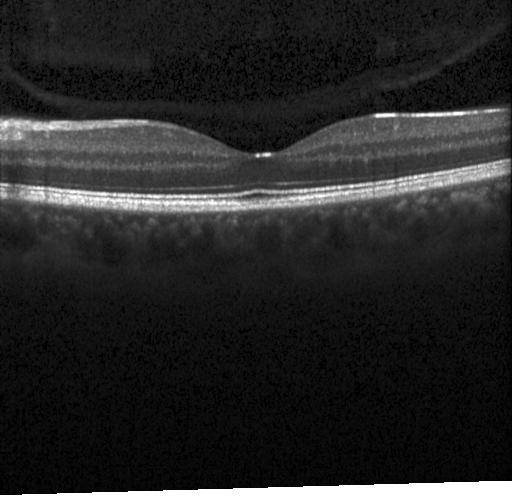 Spectral-domain OCT. Retinal OCT B-scan. Acquired on a Heidelberg Spectralis
Impression: no evidence of choroidal neovascularization, diabetic macular edema, or drusen.